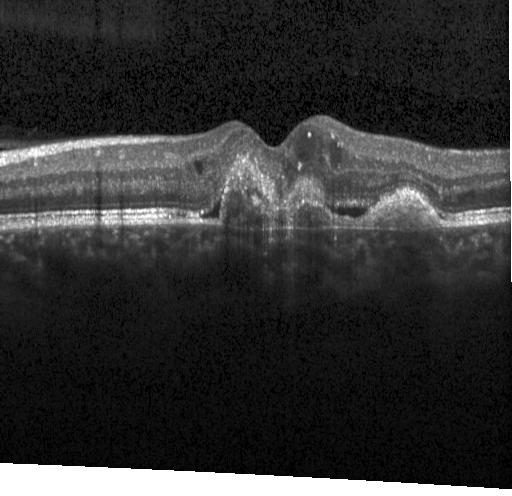 Diagnosis: a choroidal neovascular membrane.